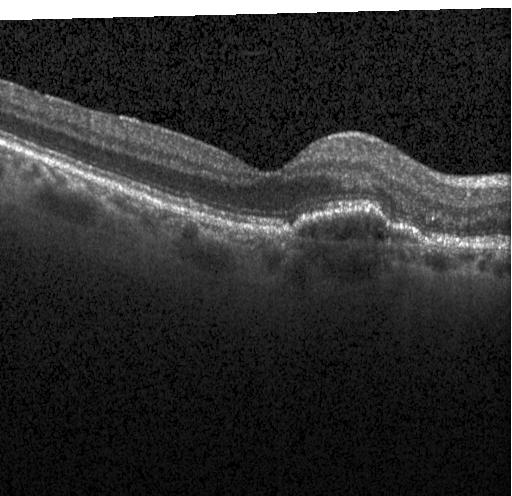
Through the macula. Retinal OCT cross-section. Heidelberg Spectralis OCT system. Spectral-domain optical coherence tomography
This B-scan demonstrates CNV.